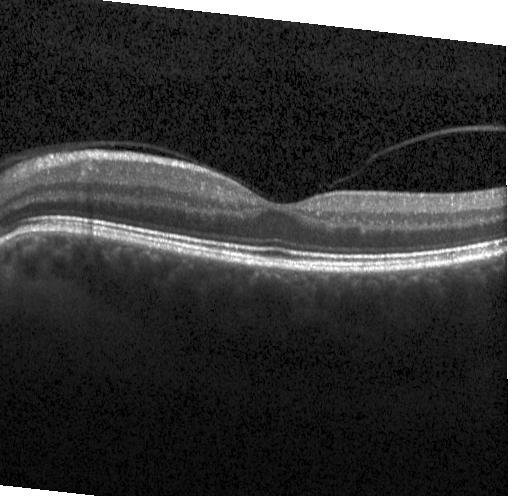

Instrument: Heidelberg Spectralis; retinal OCT cross-section; spectral-domain OCT; through the macula. OCT finding: no CNV, no DME, and no drusen.